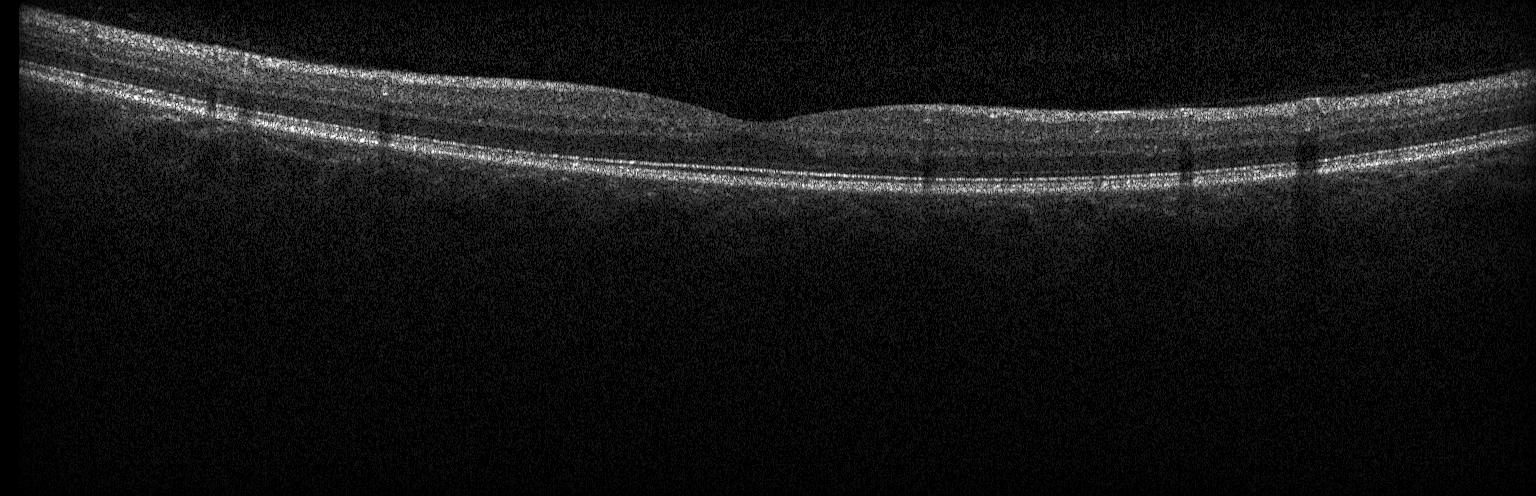 Heidelberg Spectralis OCT system, OCT line scan.
Finding: neither choroidal neovascularization, diabetic macular edema, nor drusen.